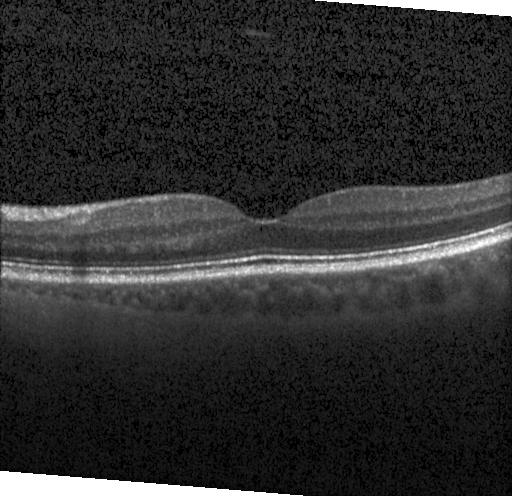

Fovea-centered; retinal OCT cross-section; spectral-domain optical coherence tomography; instrument: Heidelberg Spectralis. Neither choroidal neovascularization, diabetic macular edema, nor drusen.